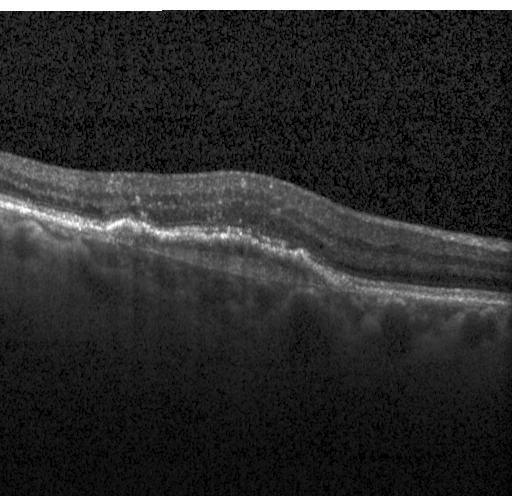 Retinal OCT B-scan
Finding: choroidal neovascularization (CNV).